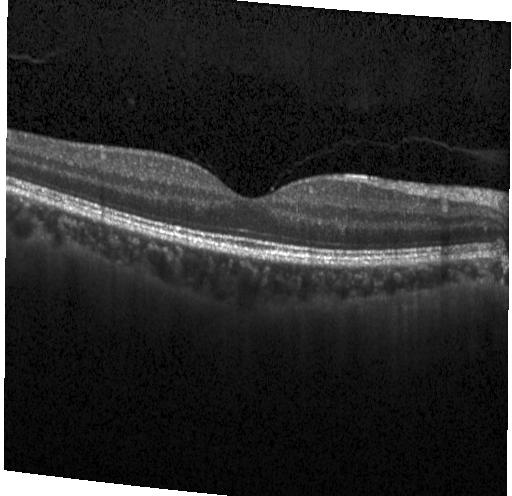 Finding: neither choroidal neovascularization, diabetic macular edema, nor drusen.